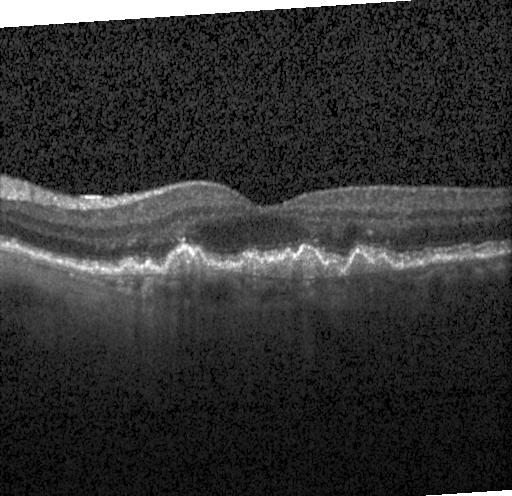 Spectral-domain OCT · optical coherence tomography scan.
Impression: multiple drusen.